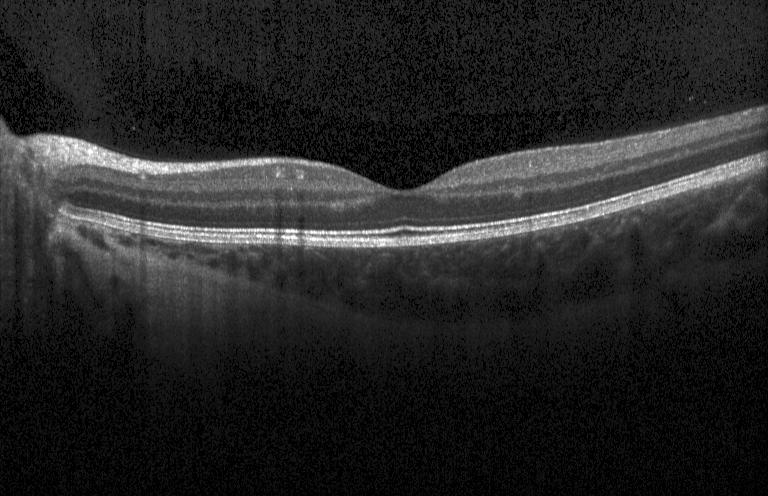

Diagnosis: no evidence of CNV, DME, or drusen.